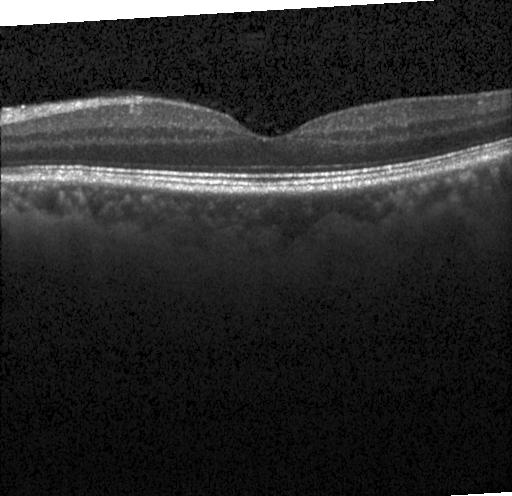 Assessment: no choroidal neovascularization, no diabetic macular edema, and no drusen.